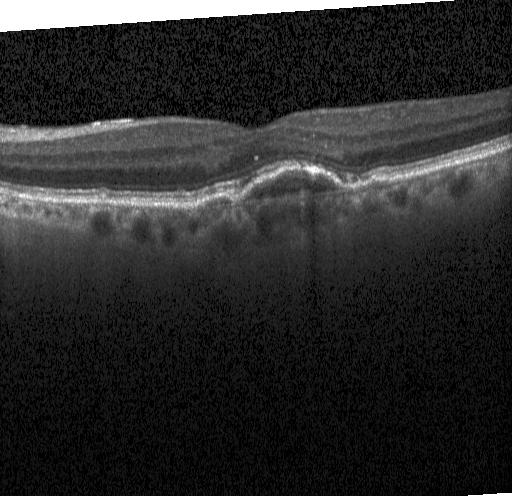 Spectral-domain optical coherence tomography. OCT line scan. Acquired on a Heidelberg Spectralis. Macular scan.
A choroidal neovascular membrane.